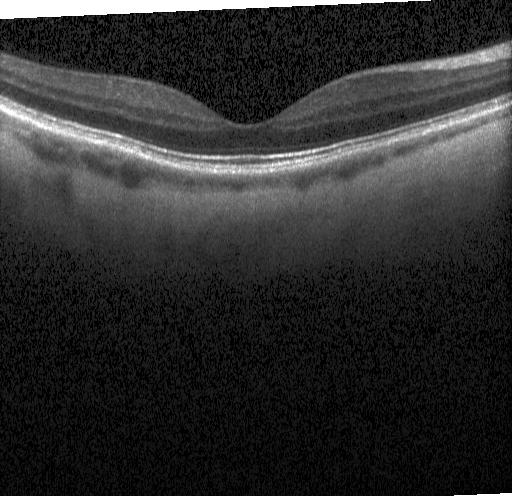
Optical coherence tomography B-scan · horizontal scan through the fovea · SD-OCT.
The scan shows neither choroidal neovascularization, diabetic macular edema, nor drusen.